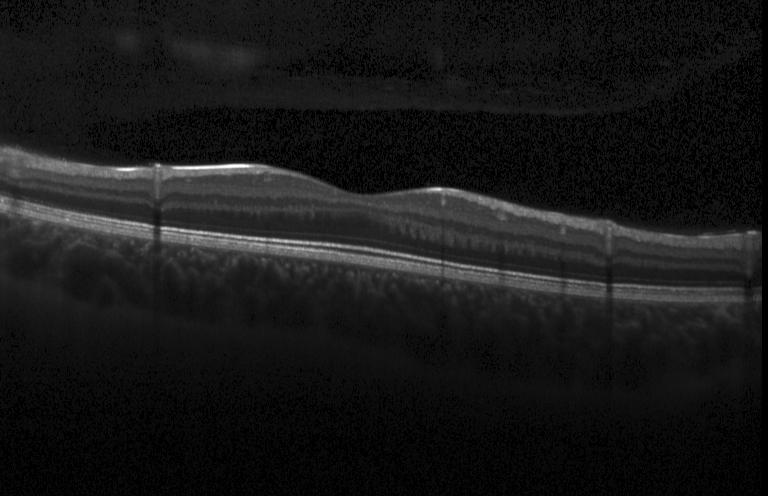 Retinal OCT cross-section. Heidelberg Spectralis OCT system. SD-OCT. Macular scan.
OCT finding: neither choroidal neovascularization, diabetic macular edema, nor drusen.